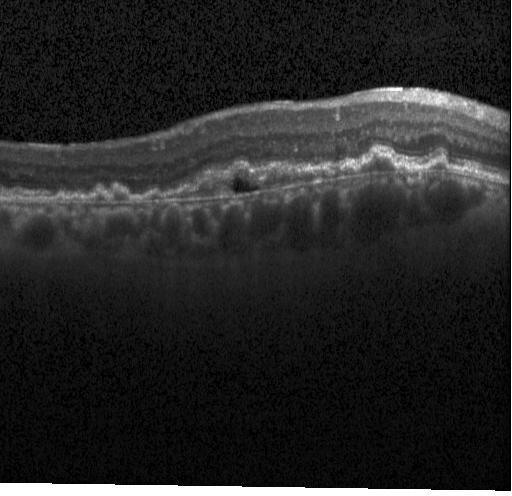 Heidelberg Spectralis. SD-OCT. OCT B-scan. Fovea-centered.
Impression: a choroidal neovascular membrane.